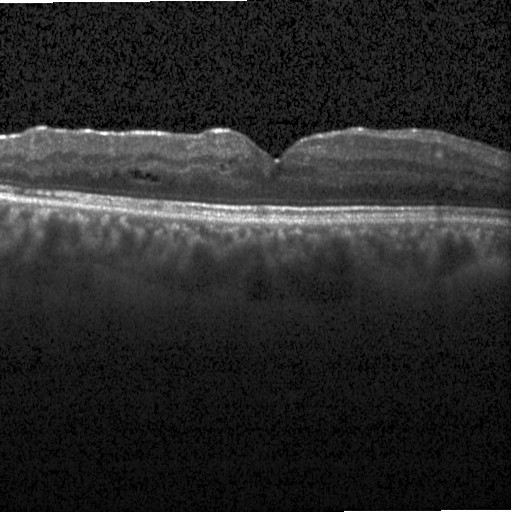

OCT B-scan; Heidelberg Spectralis OCT system; spectral-domain optical coherence tomography
Impression: diabetic macular edema.